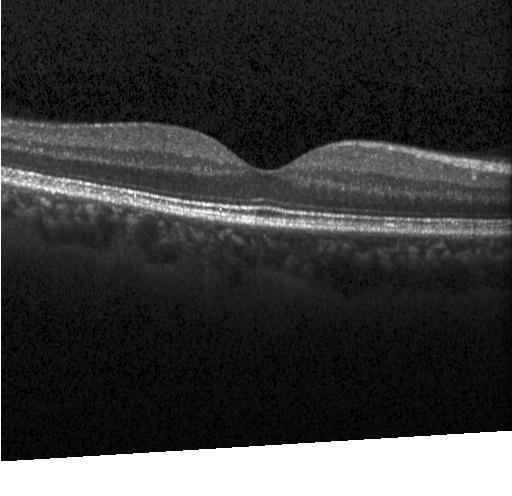
Optical coherence tomography scan, spectral-domain OCT, Heidelberg Spectralis, fovea-centered
No choroidal neovascularization, no diabetic macular edema, and no drusen.